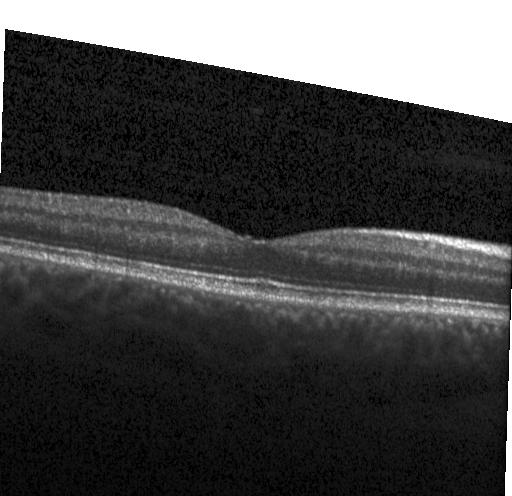
Instrument: Heidelberg Spectralis; SD-OCT; optical coherence tomography scan; macular scan.
Impression: no evidence of choroidal neovascularization, diabetic macular edema, or drusen.